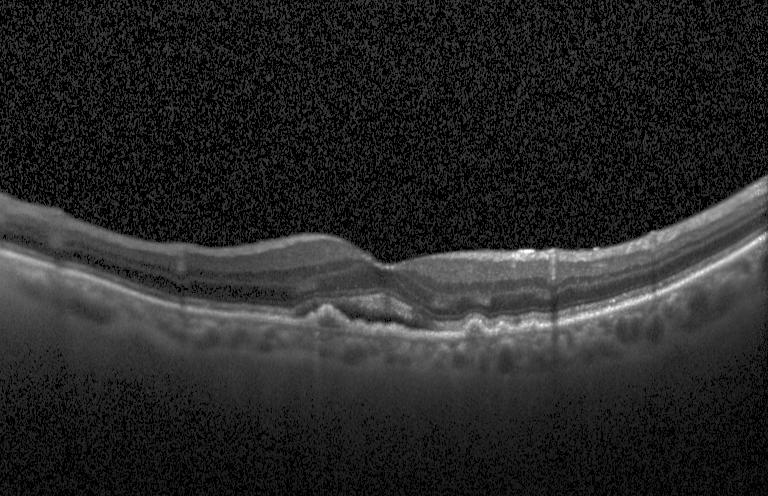 SD-OCT; fovea-centered; instrument: Heidelberg Spectralis; optical coherence tomography scan — Finding: choroidal neovascularization.